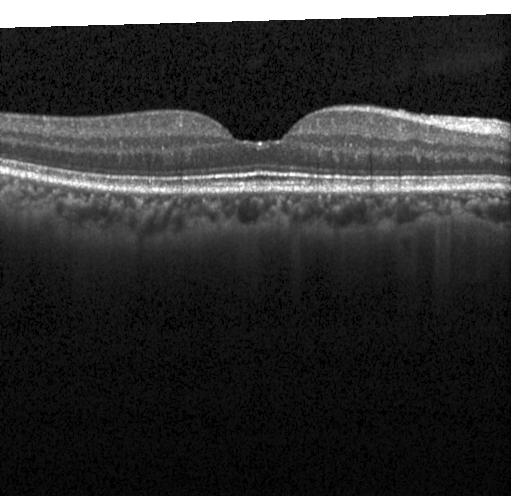

OCT scan showing no evidence of choroidal neovascularization, diabetic macular edema, or drusen.